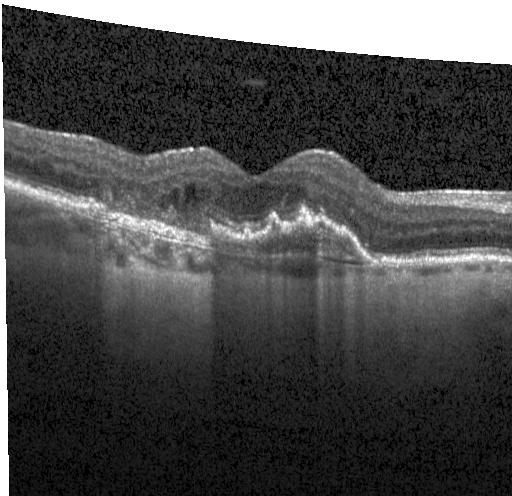

Diagnosis: a choroidal neovascular membrane.